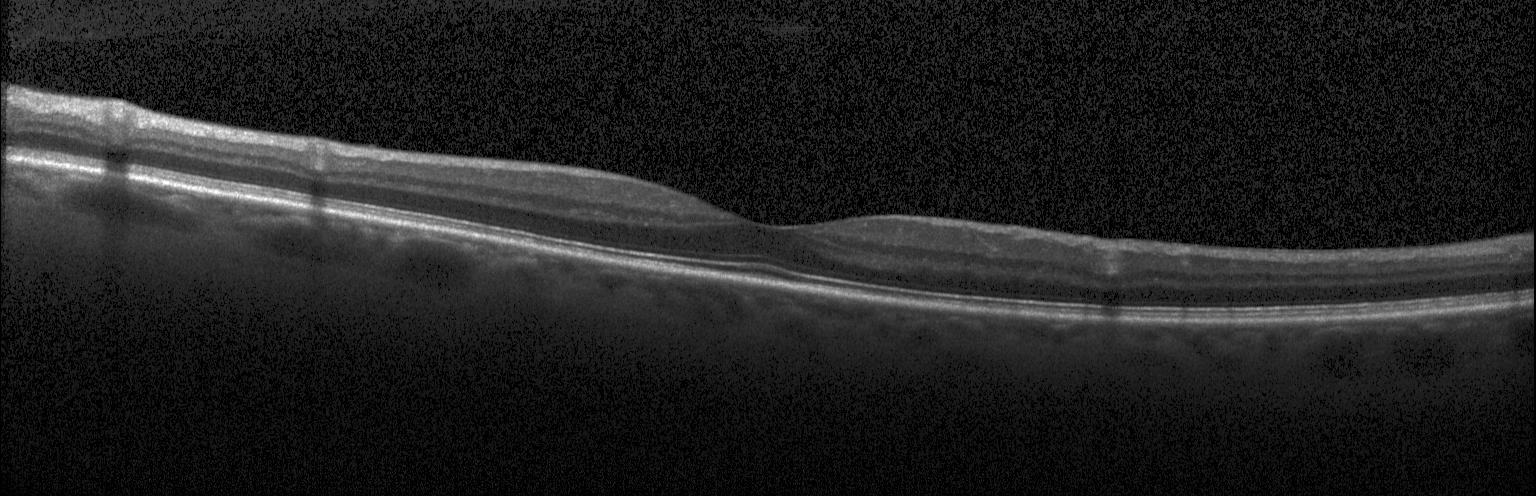
Diagnosis: no choroidal neovascularization, no diabetic macular edema, and no drusen.